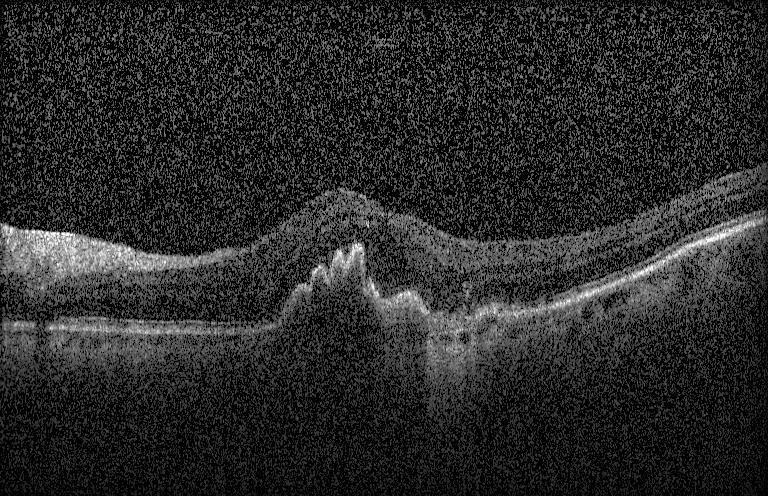 OCT scan showing CNV.